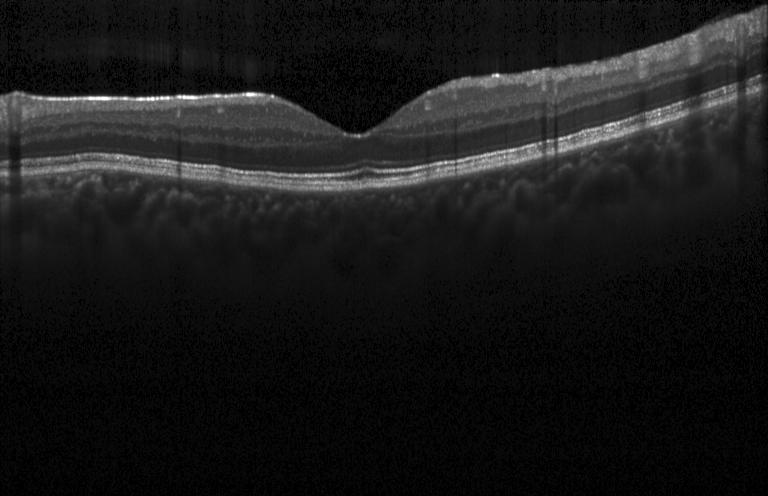
OCT line scan, through the macula — Impression: neither choroidal neovascularization, diabetic macular edema, nor drusen.